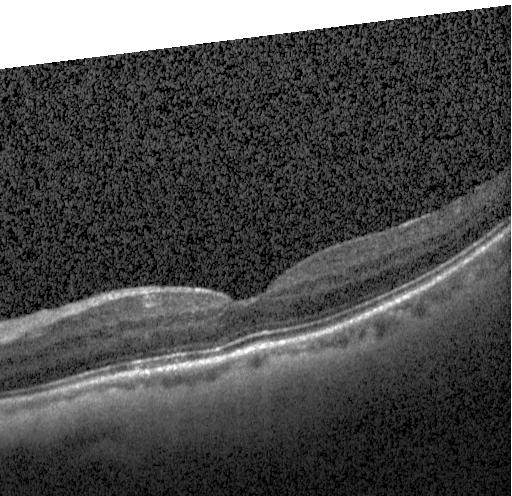
Finding: neither CNV, DME, nor drusen.